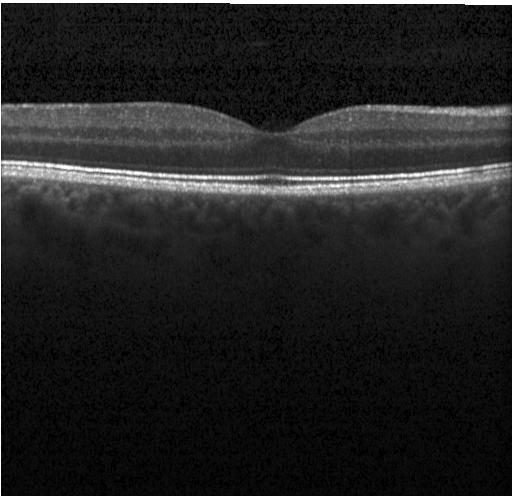
The scan shows no evidence of CNV, DME, or drusen.